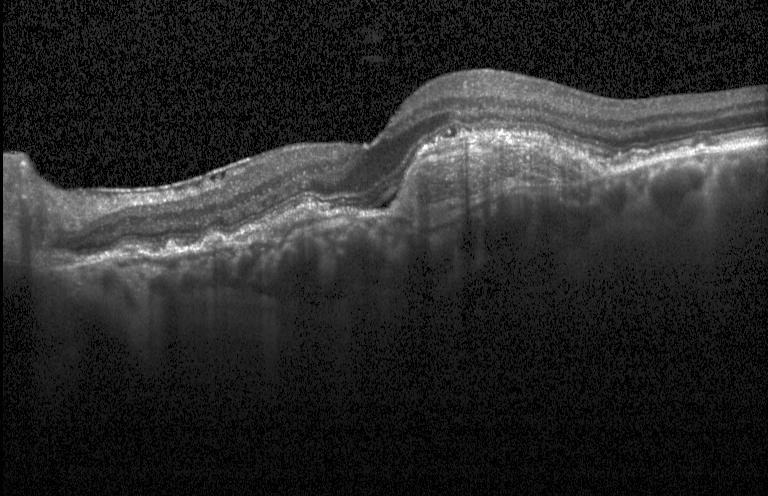
Optical coherence tomography scan, acquired on a Heidelberg Spectralis, spectral-domain optical coherence tomography, fovea-centered — The scan shows a choroidal neovascular membrane.